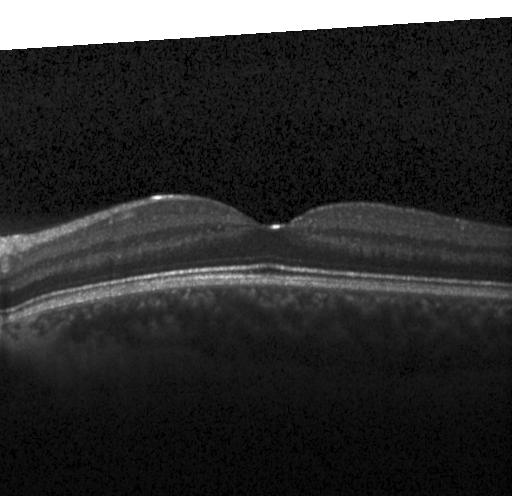 Retinal OCT B-scan · through the macula — Diagnosis: no CNV, no DME, and no drusen.